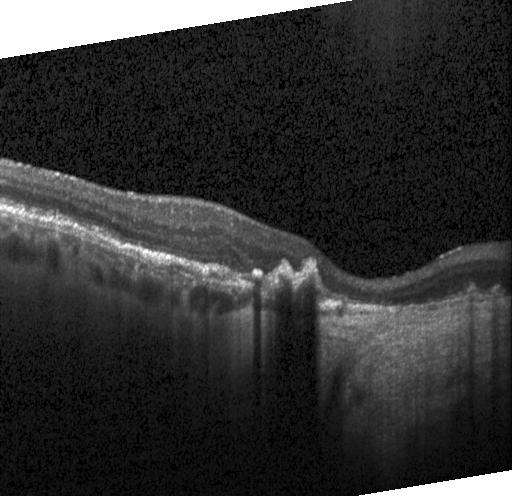

Through the macula. Acquired on a Heidelberg Spectralis. Retinal OCT cross-section. Spectral-domain OCT.
A choroidal neovascular membrane.